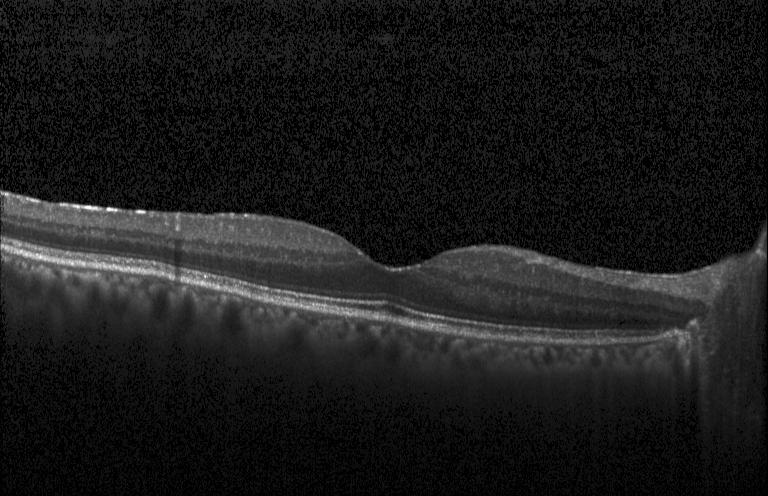
Optical coherence tomography B-scan
Diagnosis: no choroidal neovascularization, no diabetic macular edema, and no drusen.